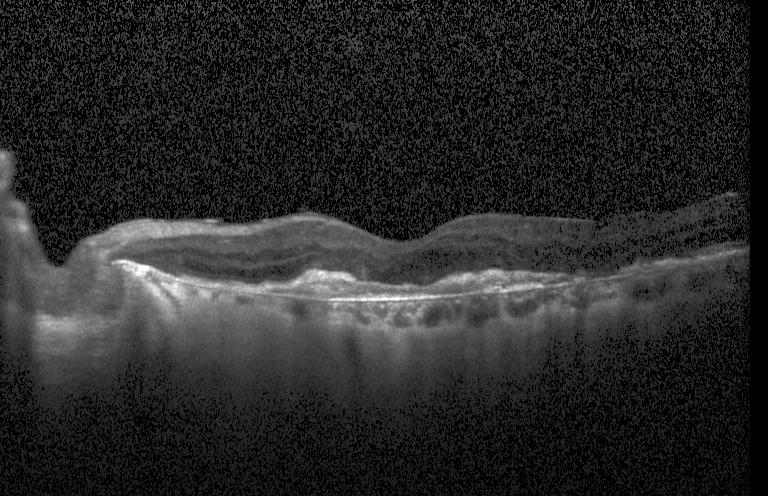 Macular scan · SD-OCT · retinal OCT B-scan · acquired on a Heidelberg Spectralis — Impression: a choroidal neovascular membrane.